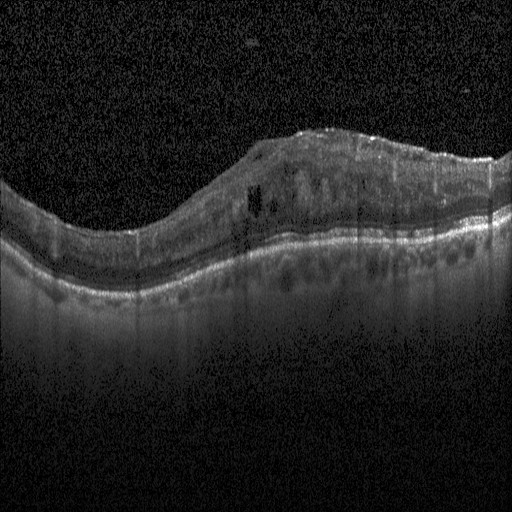
Optical coherence tomography scan; spectral-domain optical coherence tomography
Finding: diabetic macular edema (DME).